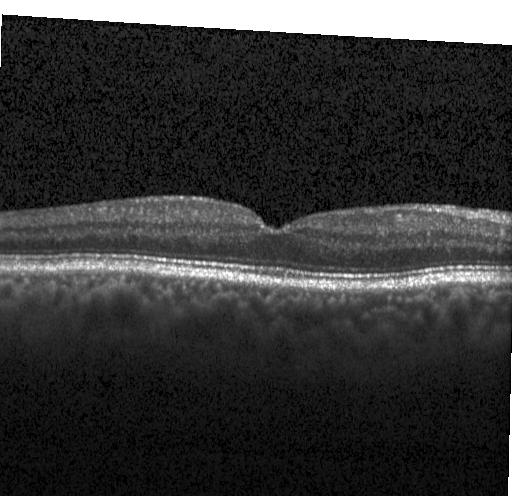
Retinal OCT B-scan; SD-OCT; through the macula. Impression: no evidence of choroidal neovascularization, diabetic macular edema, or drusen.